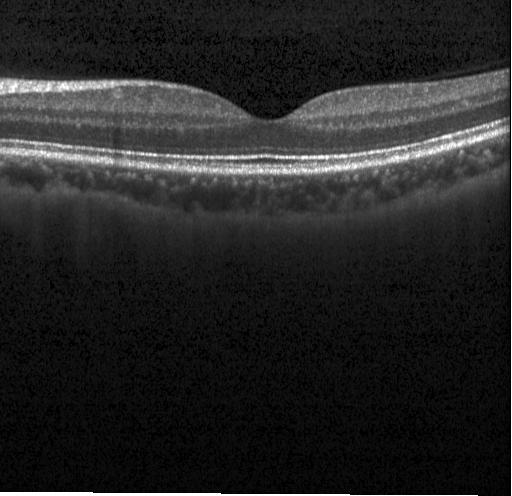 Spectral-domain OCT · horizontal scan through the fovea · instrument: Heidelberg Spectralis · retinal OCT B-scan.
Finding: no evidence of CNV, DME, or drusen.